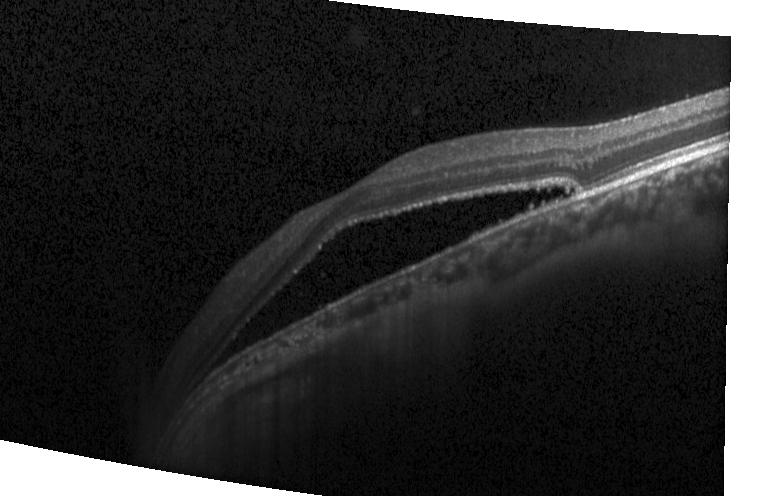 Acquired on a Heidelberg Spectralis; SD-OCT; OCT line scan.
CNV.